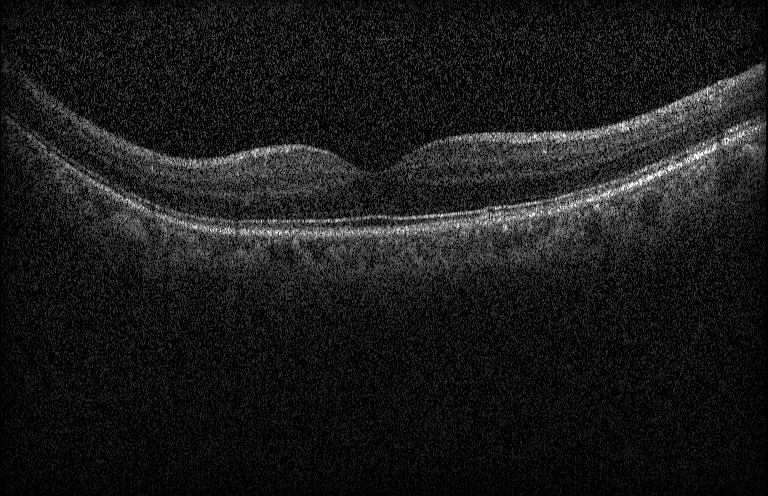 Diagnosis: neither choroidal neovascularization, diabetic macular edema, nor drusen.